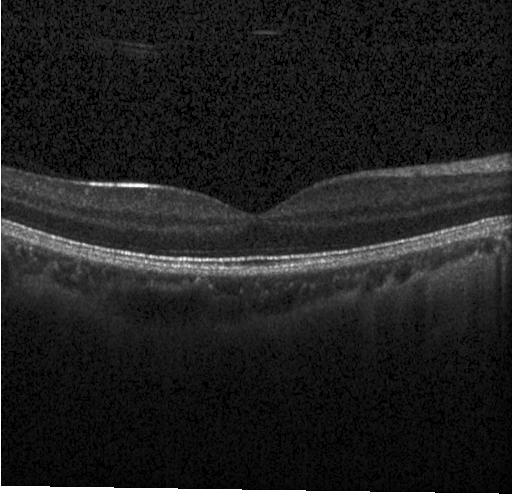
Finding: no CNV, DME, or drusen.